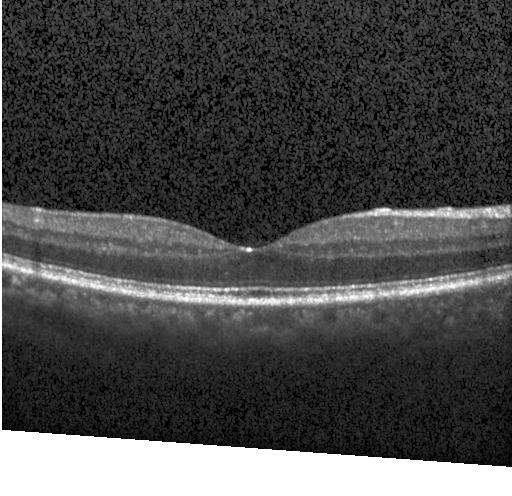
Finding: no choroidal neovascularization, no diabetic macular edema, and no drusen.